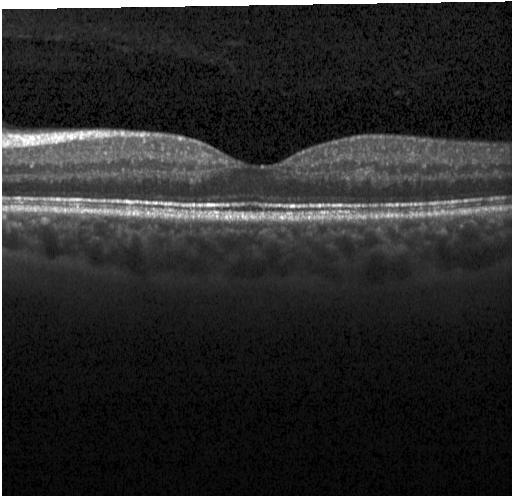

OCT scan showing no choroidal neovascularization, no diabetic macular edema, and no drusen.